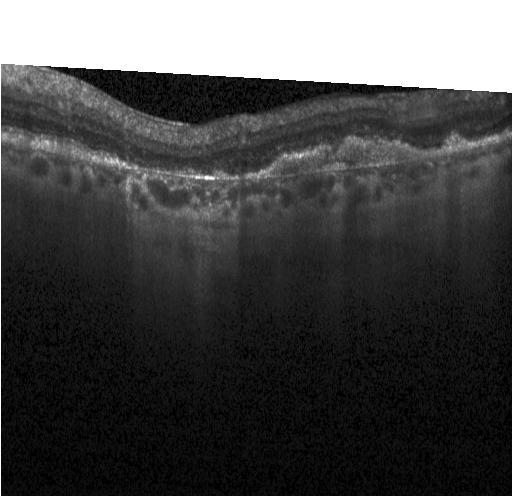
The scan shows a choroidal neovascular membrane.